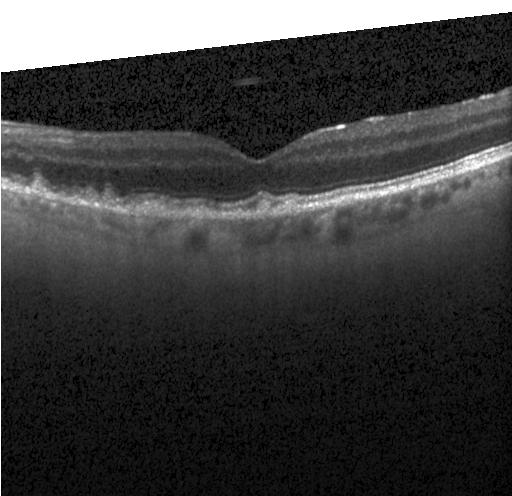 Instrument: Heidelberg Spectralis · centered on the fovea · OCT line scan — Finding: multiple drusen.